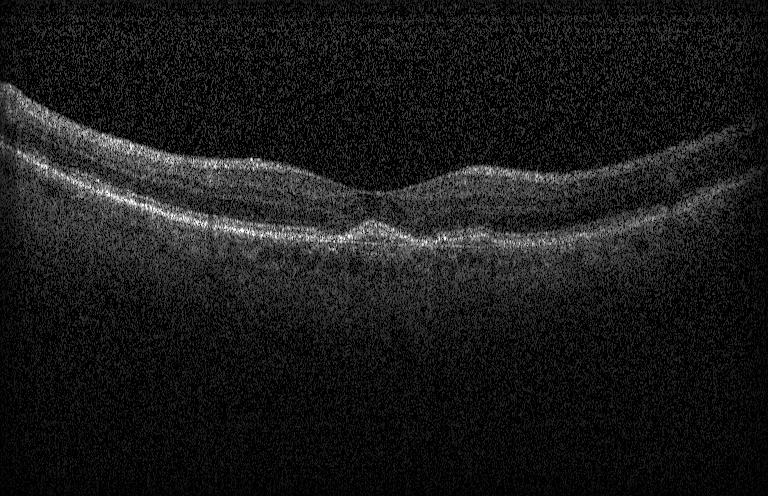
Through the macula, spectral-domain optical coherence tomography, acquired on a Heidelberg Spectralis, OCT B-scan. OCT finding: choroidal neovascularization (CNV).